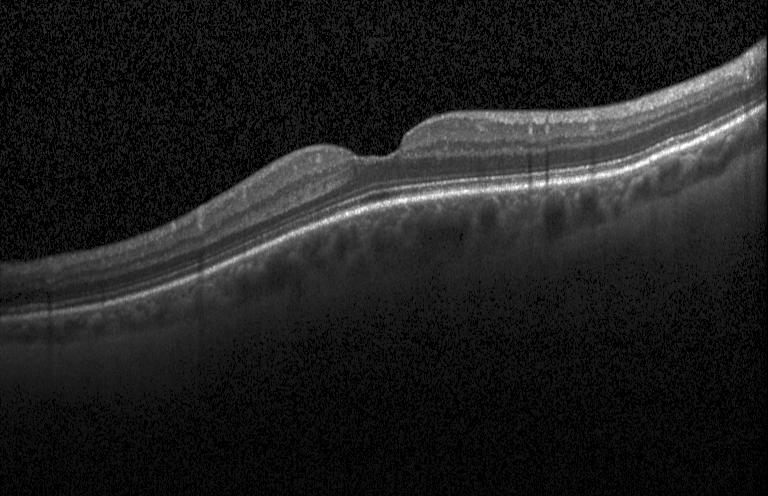
Optical coherence tomography B-scan · spectral-domain optical coherence tomography
Diagnosis: neither choroidal neovascularization, diabetic macular edema, nor drusen.